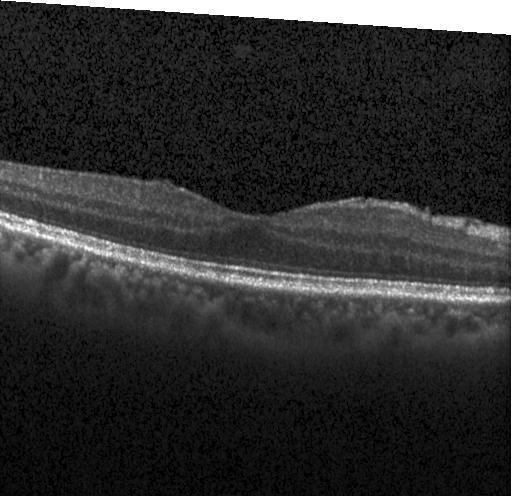 Horizontal scan through the fovea, Heidelberg Spectralis, OCT B-scan, SD-OCT
Impression: no choroidal neovascularization, diabetic macular edema, or drusen.